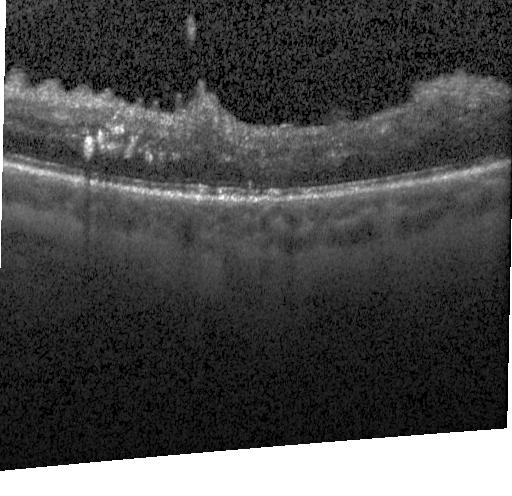 Heidelberg Spectralis, macular scan, spectral-domain OCT, retinal OCT B-scan. Impression: diabetic macular edema (DME).